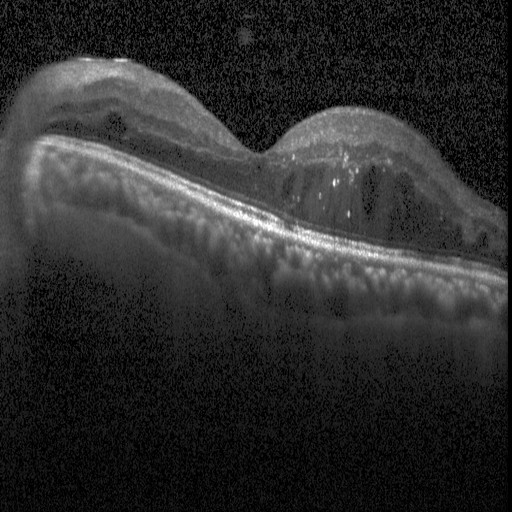
This B-scan demonstrates DME.